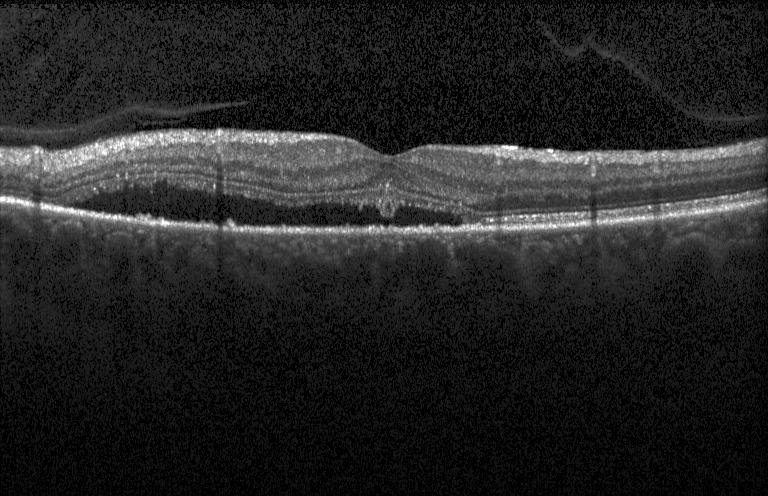 This B-scan demonstrates a choroidal neovascular membrane.